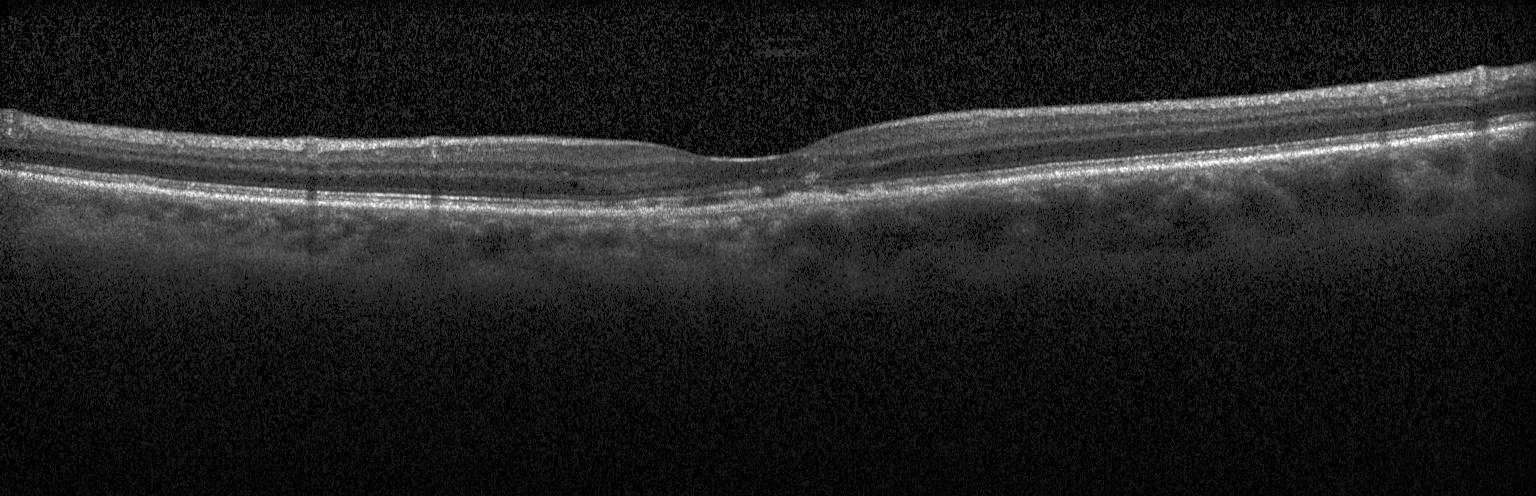

Retinal OCT cross-section. Heidelberg Spectralis OCT system. Horizontal scan through the fovea. SD-OCT. CNV.